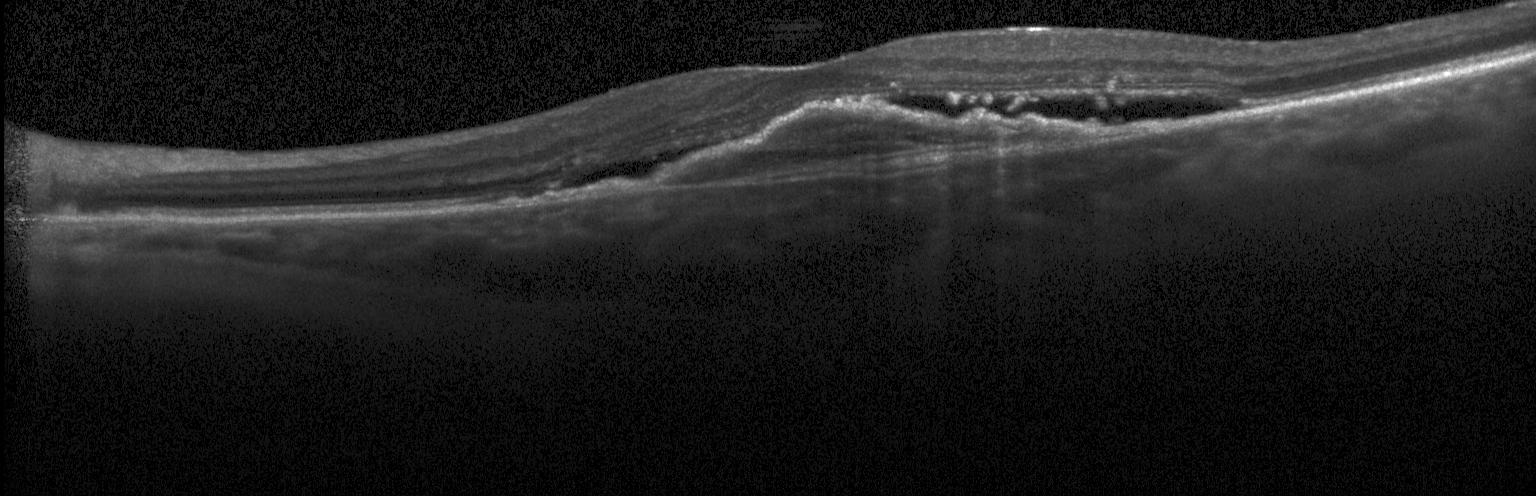

Through the macula; spectral-domain OCT; acquired on a Heidelberg Spectralis; OCT B-scan — Assessment: CNV.